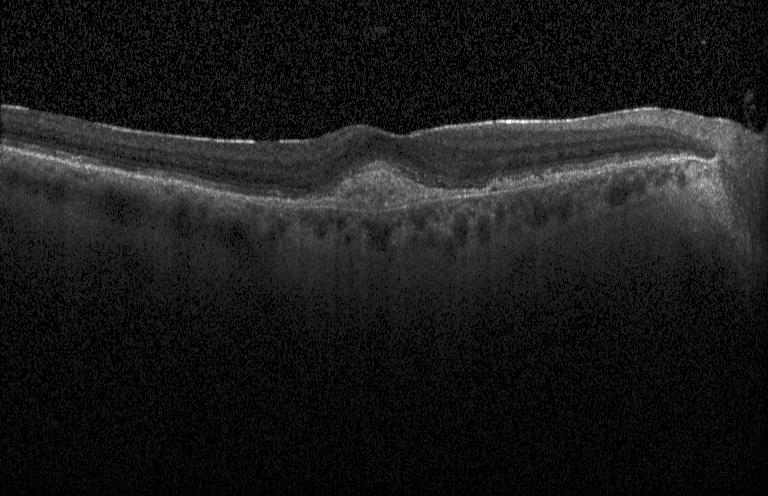
Diagnosis: choroidal neovascularization.